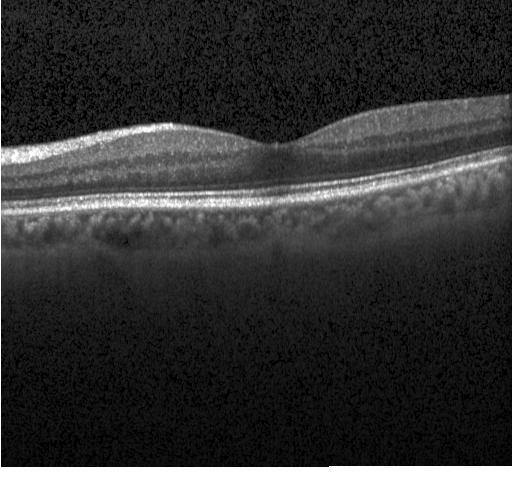
Macular OCT: neither choroidal neovascularization, diabetic macular edema, nor drusen.